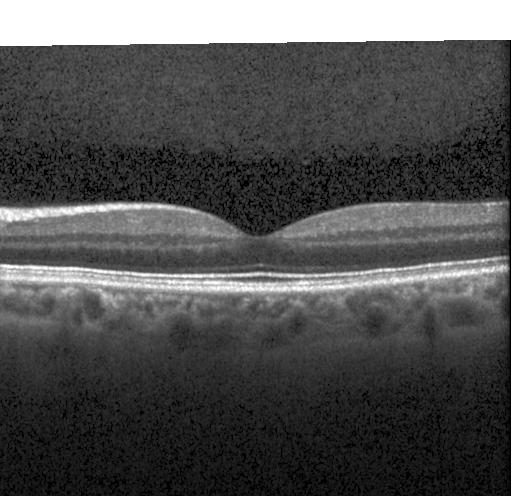

OCT scan showing no choroidal neovascularization, diabetic macular edema, or drusen.